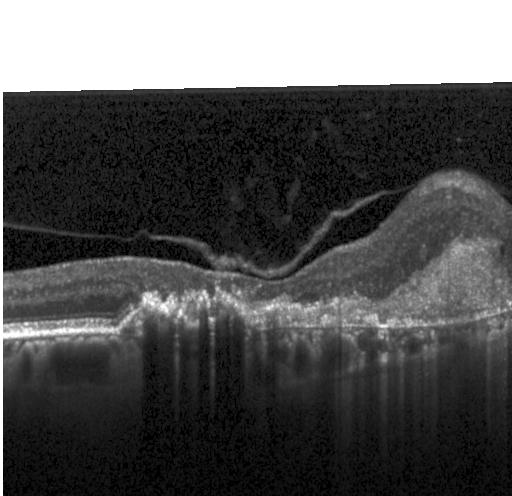
Optical coherence tomography B-scan. Centered on the fovea. SD-OCT. Acquired on a Heidelberg Spectralis — This B-scan demonstrates choroidal neovascularization (CNV).